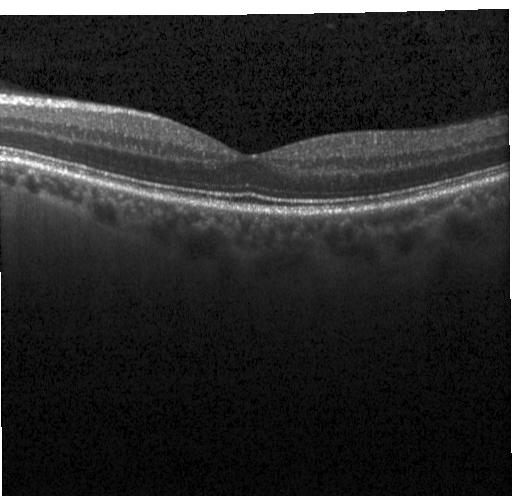
OCT finding: no evidence of choroidal neovascularization, diabetic macular edema, or drusen.